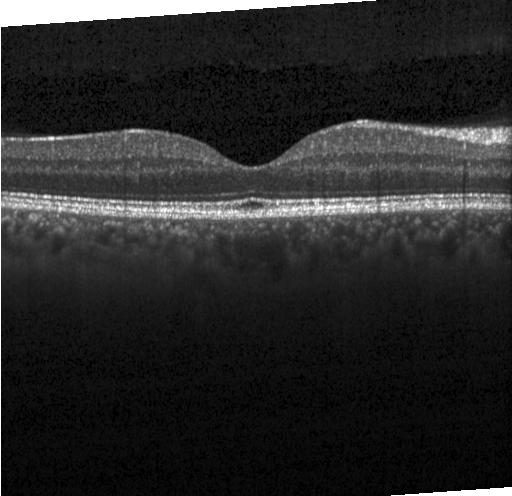
Spectral-domain OCT; optical coherence tomography scan; fovea-centered; acquired on a Heidelberg Spectralis.
Finding: no evidence of choroidal neovascularization, diabetic macular edema, or drusen.